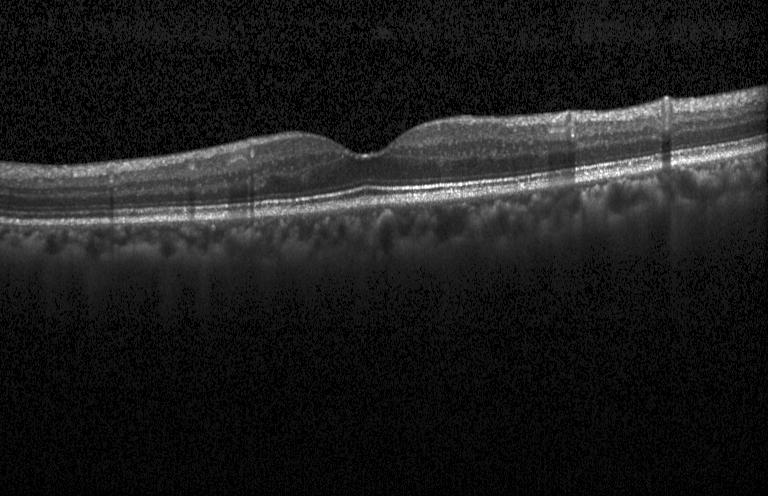

No evidence of choroidal neovascularization, diabetic macular edema, or drusen.